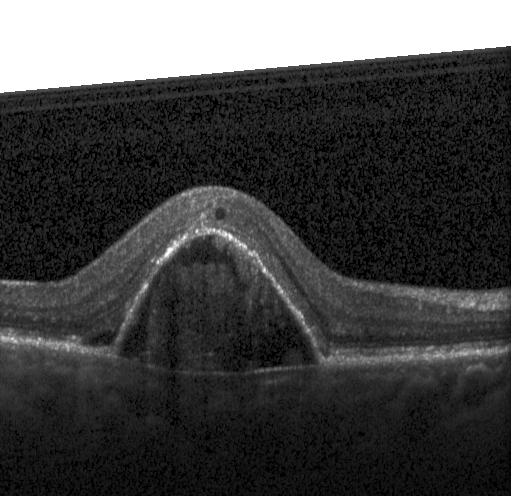
OCT line scan. Instrument: Heidelberg Spectralis. Dx: a choroidal neovascular membrane.